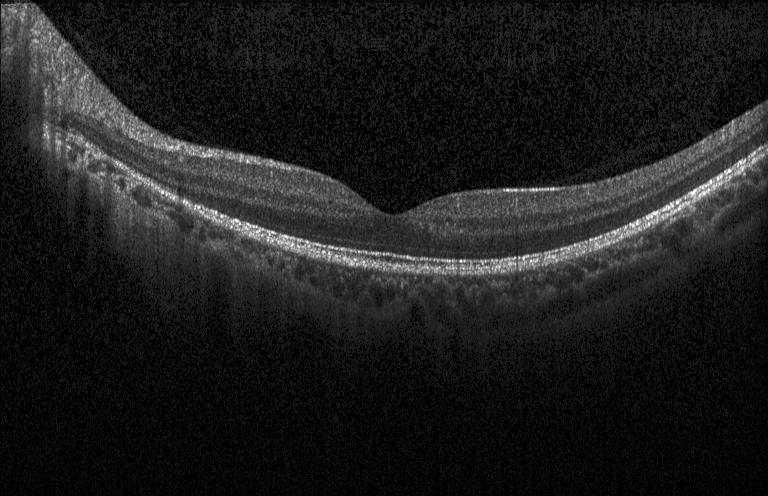

Optical coherence tomography scan; SD-OCT. Diagnosis: no evidence of CNV, DME, or drusen.